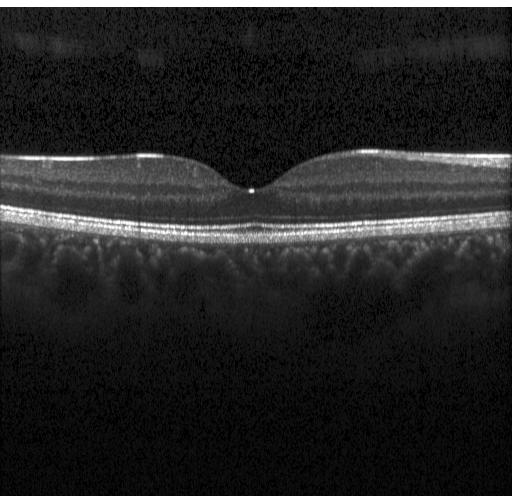 OCT finding: no choroidal neovascularization, diabetic macular edema, or drusen.